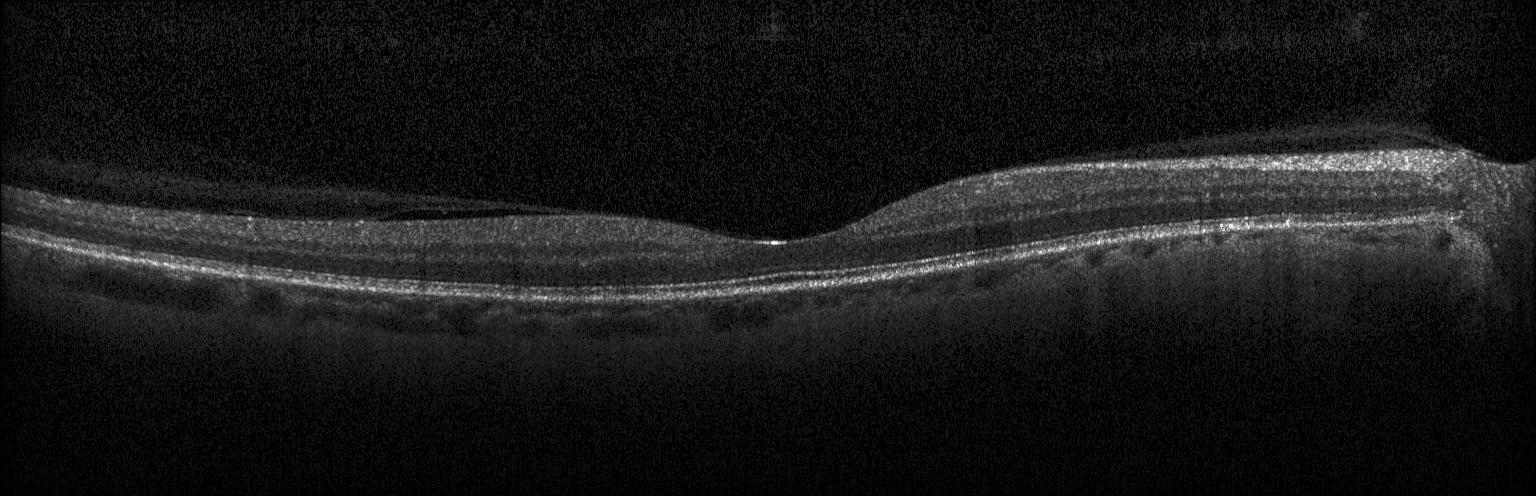
Optical coherence tomography B-scan · Heidelberg Spectralis.
Finding: neither choroidal neovascularization, diabetic macular edema, nor drusen.